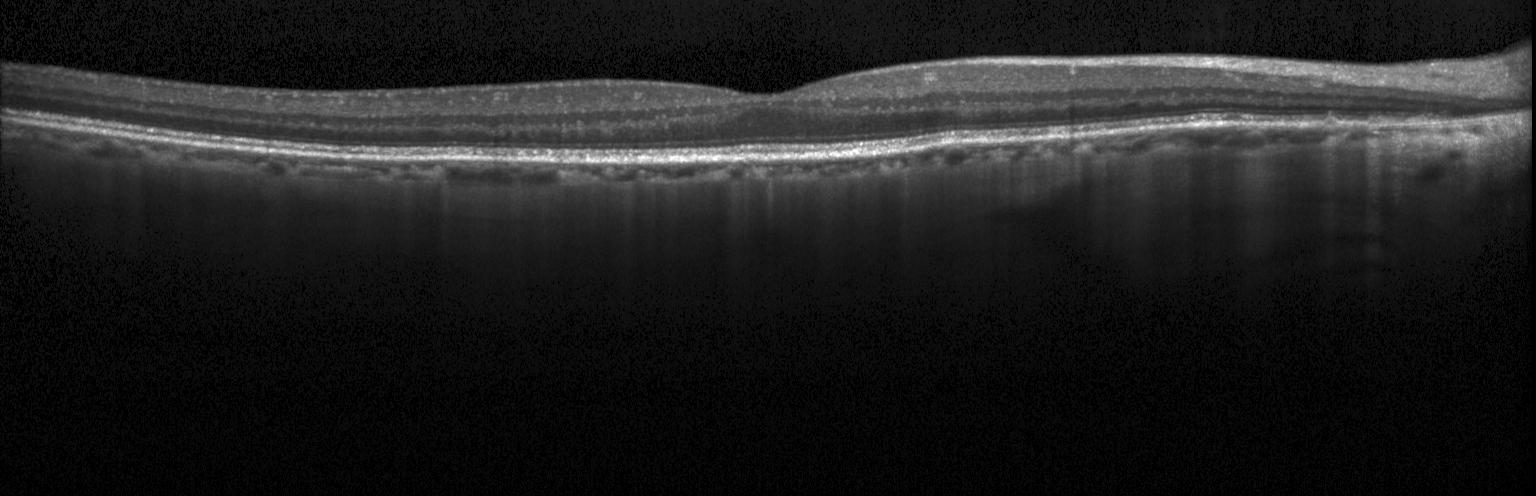

OCT B-scan · spectral-domain OCT. Diagnosis: neither choroidal neovascularization, diabetic macular edema, nor drusen.